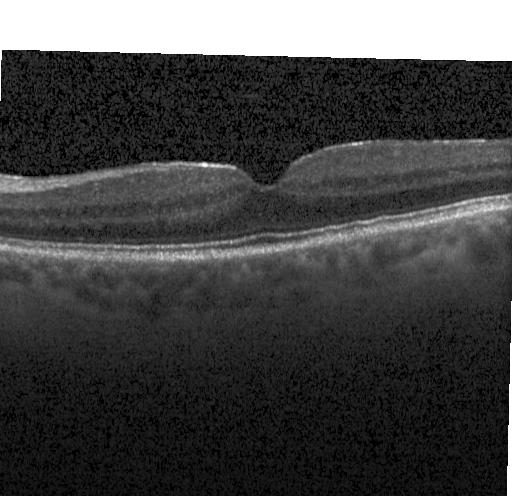 Assessment: no choroidal neovascularization, no diabetic macular edema, and no drusen.